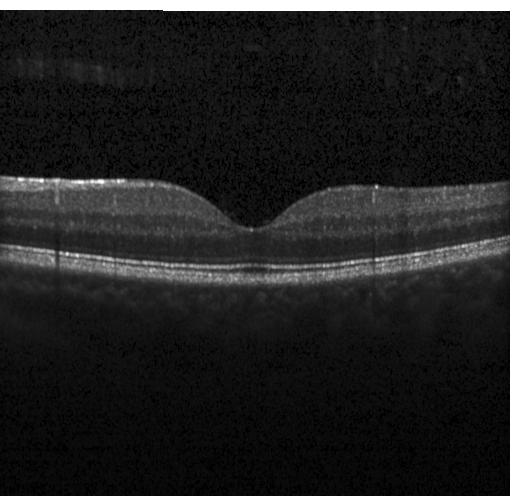 Retinal OCT B-scan
Assessment: no evidence of choroidal neovascularization, diabetic macular edema, or drusen.